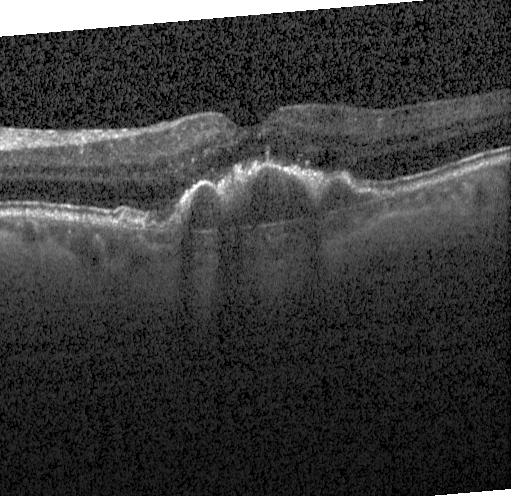 Diagnosis: choroidal neovascularization.